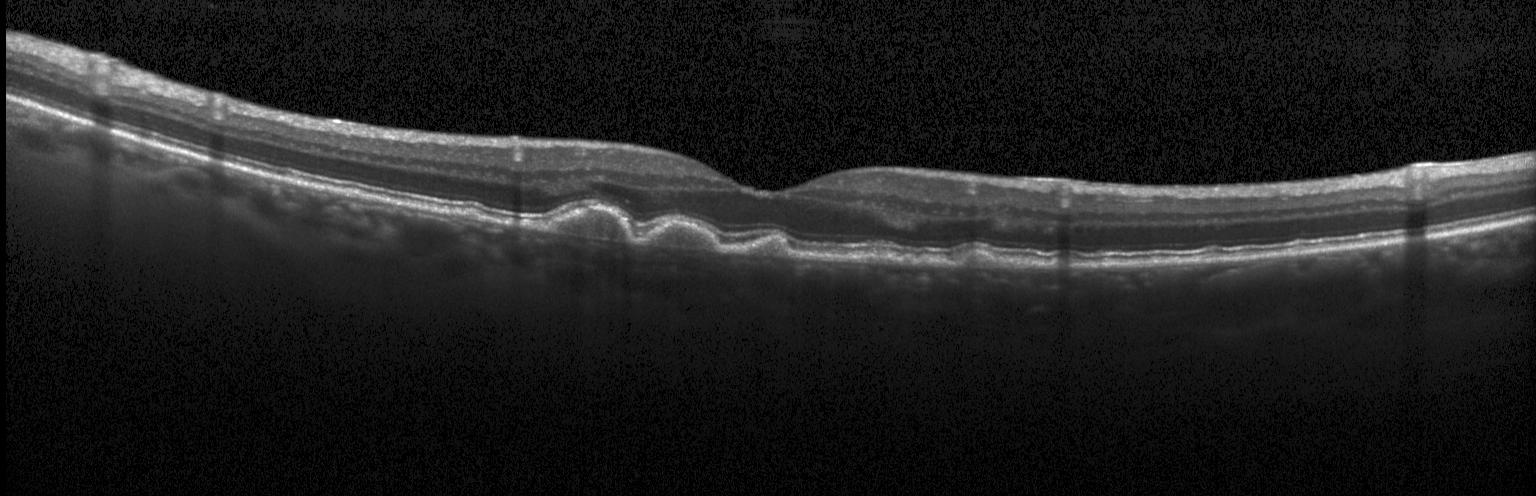 Dx: multiple drusen.